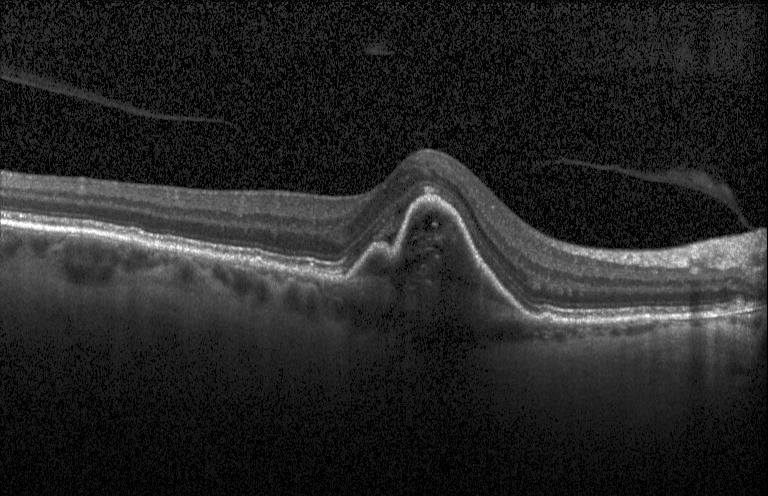 Dx: choroidal neovascularization.